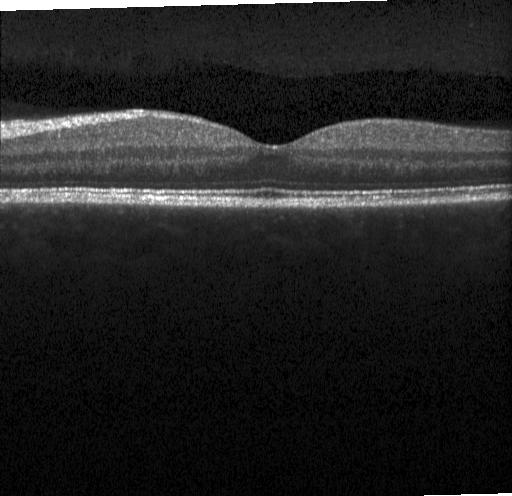

The scan shows no evidence of choroidal neovascularization, diabetic macular edema, or drusen.